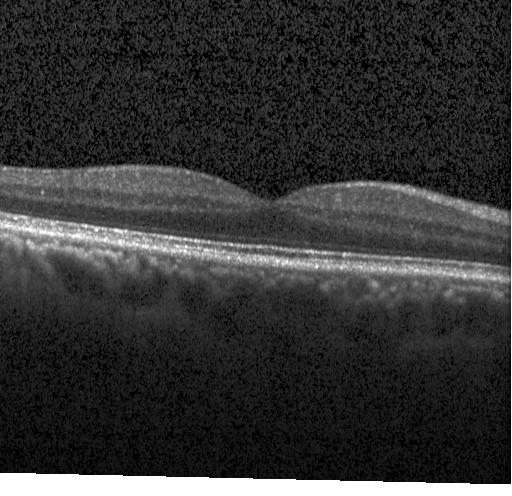

Optical coherence tomography B-scan.
Diagnosis: no CNV, DME, or drusen.